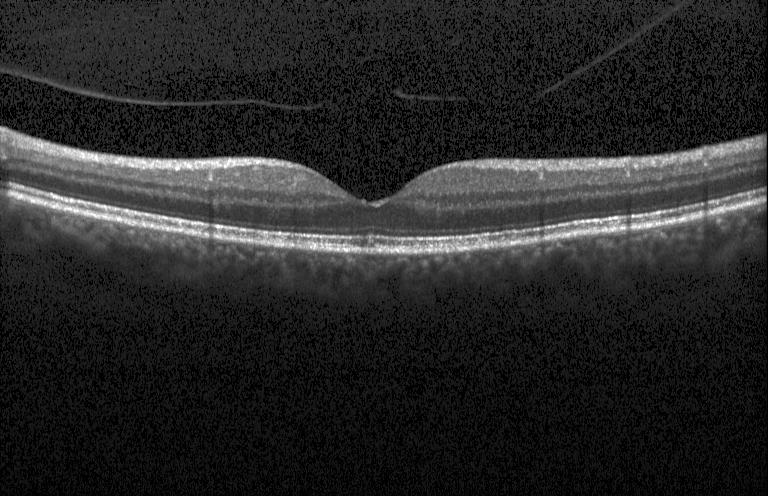
Assessment: neither choroidal neovascularization, diabetic macular edema, nor drusen.